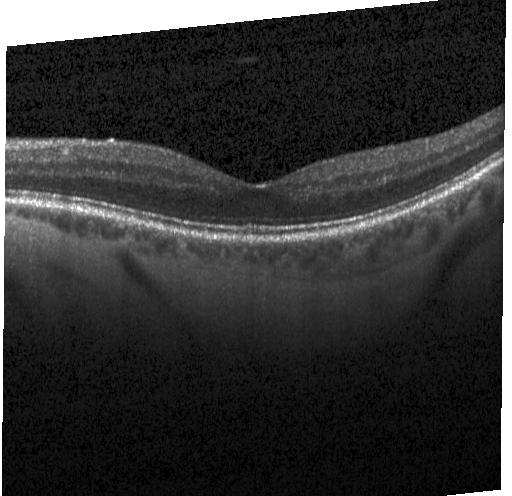

Centered on the fovea, optical coherence tomography B-scan — Macular OCT: no choroidal neovascularization, diabetic macular edema, or drusen.